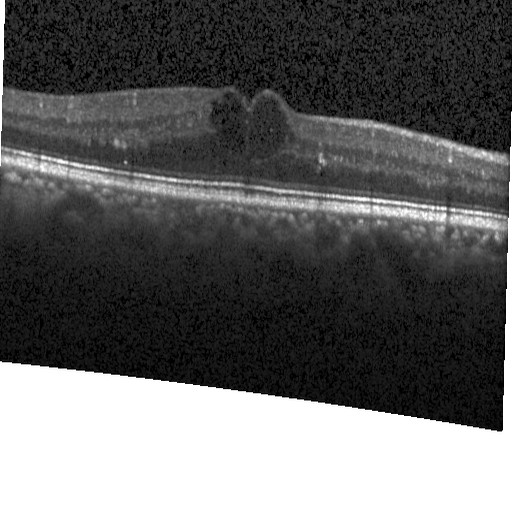 Acquired on a Heidelberg Spectralis, fovea-centered, retinal OCT B-scan, spectral-domain OCT — DME.